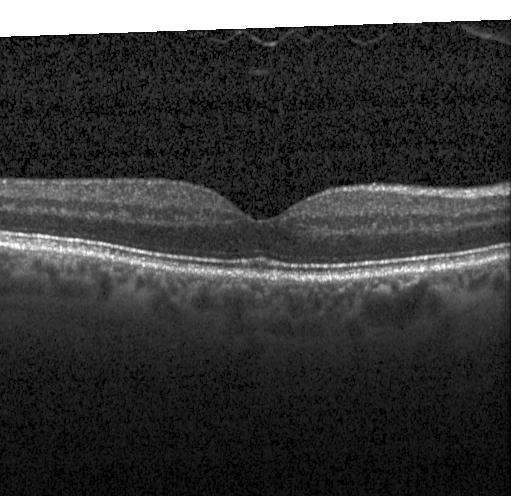 Optical coherence tomography scan, acquired on a Heidelberg Spectralis, centered on the fovea
The scan shows no choroidal neovascularization, diabetic macular edema, or drusen.